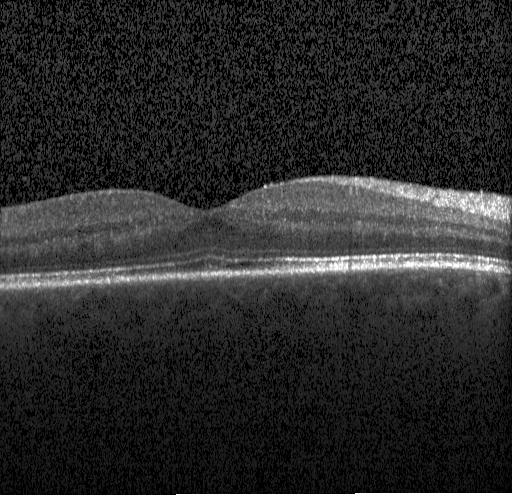
Finding: no choroidal neovascularization, diabetic macular edema, or drusen.